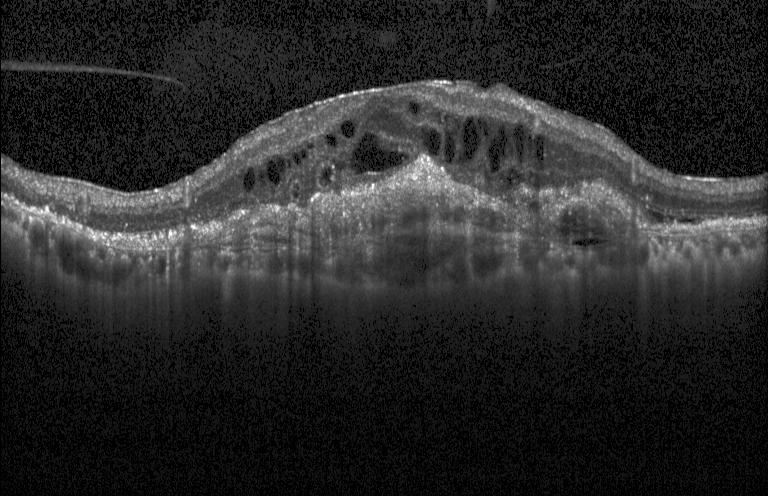
Heidelberg Spectralis OCT system. OCT B-scan. Fovea-centered. SD-OCT
Diagnosis: CNV.